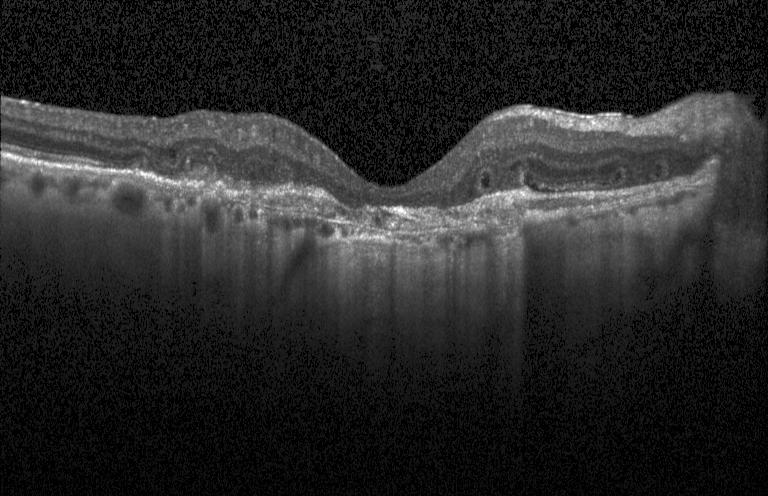 Optical coherence tomography B-scan
A choroidal neovascular membrane.